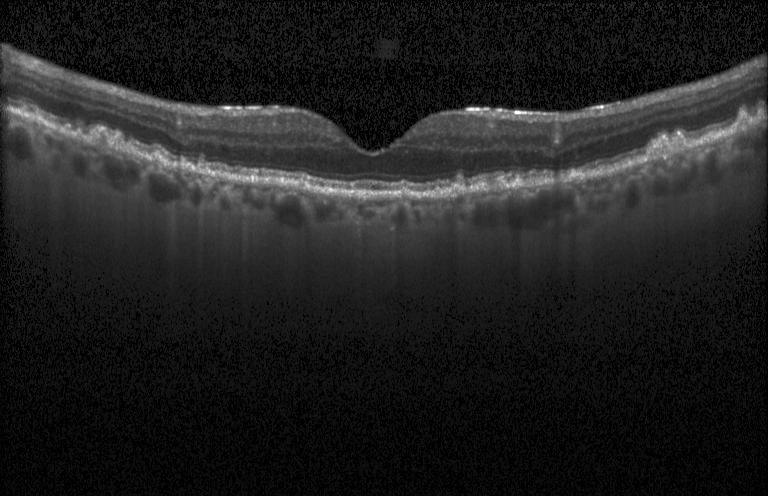 Retinal OCT cross-section; SD-OCT; through the macula — OCT finding: multiple drusen.